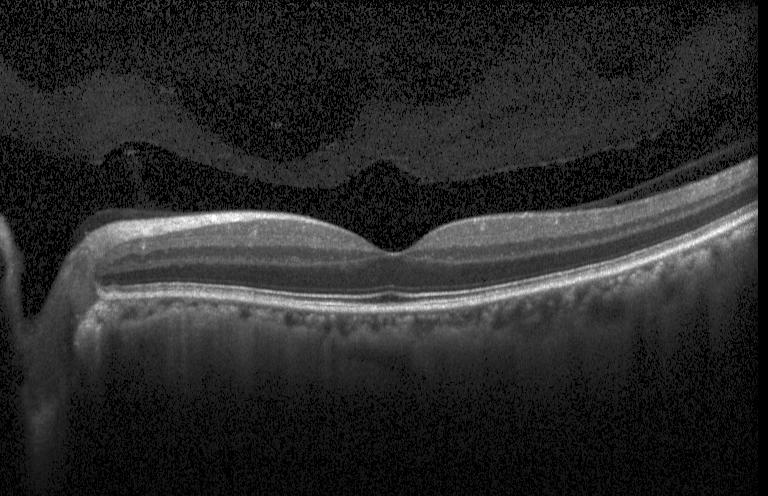

Optical coherence tomography B-scan; acquired on a Heidelberg Spectralis; spectral-domain optical coherence tomography. Macular OCT: no choroidal neovascularization, no diabetic macular edema, and no drusen.